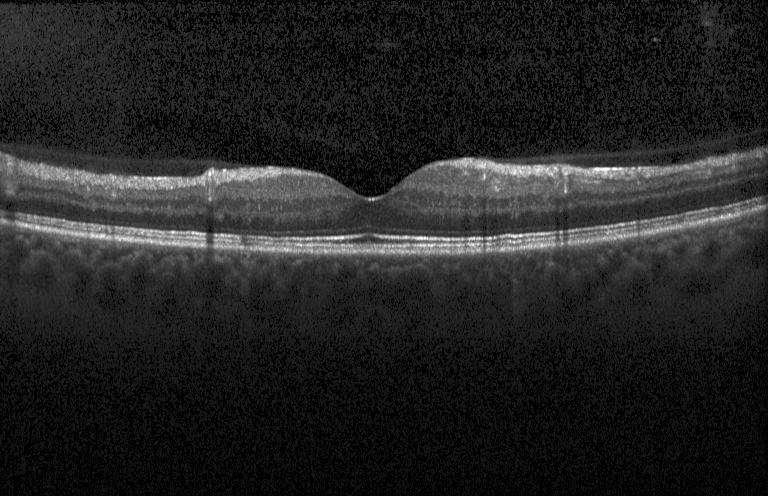 Retinal OCT cross-section.
No choroidal neovascularization, diabetic macular edema, or drusen.